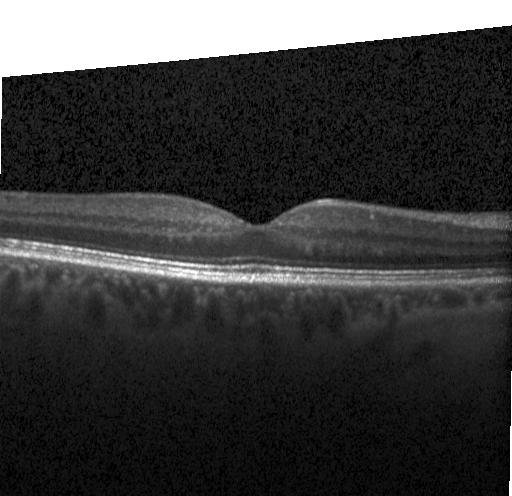

Macular OCT: no evidence of choroidal neovascularization, diabetic macular edema, or drusen.